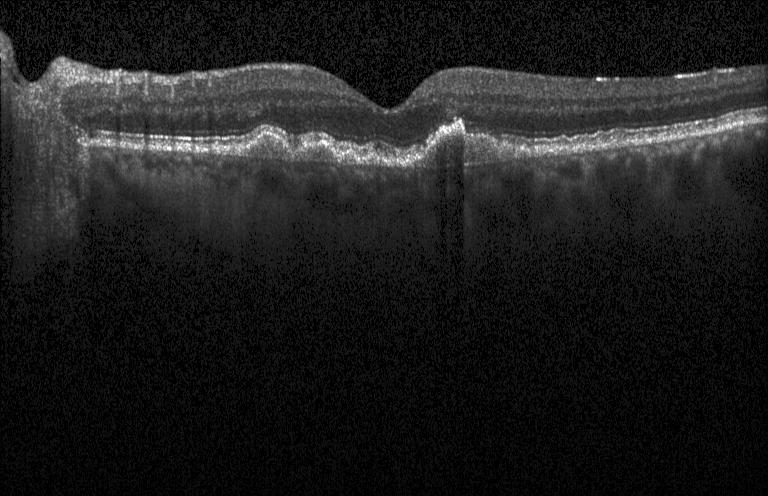

SD-OCT; optical coherence tomography B-scan. This B-scan demonstrates multiple drusen.